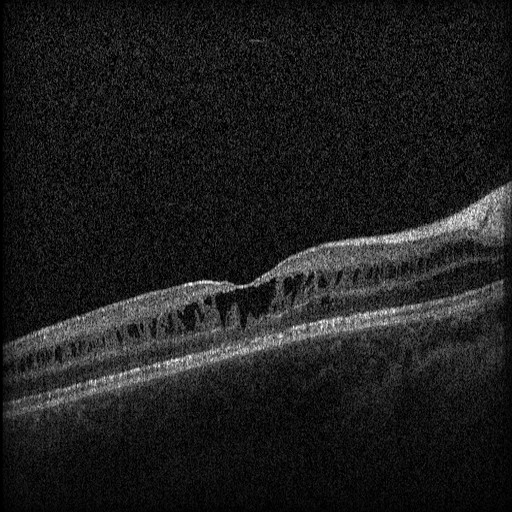 Impression: diabetic macular edema.